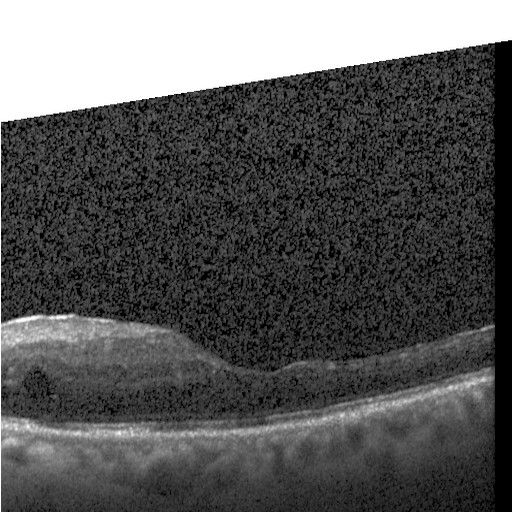

Optical coherence tomography B-scan — Finding: diabetic macular edema (DME).